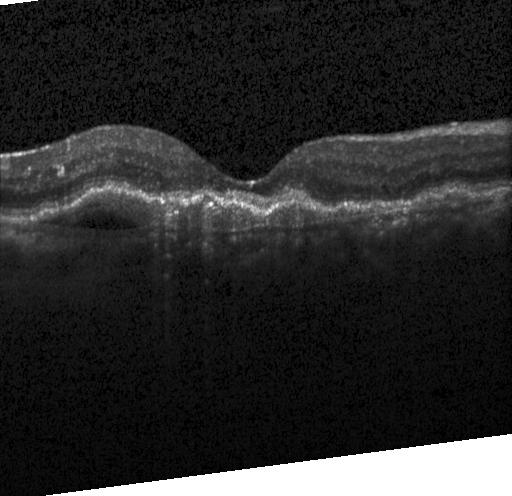
OCT scan showing a choroidal neovascular membrane.